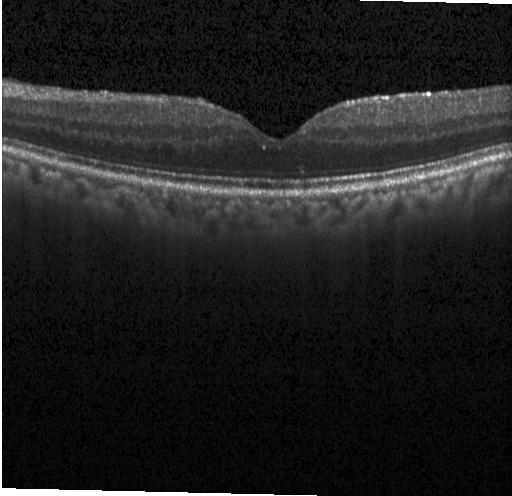

Spectral-domain OCT · retinal OCT cross-section. Impression: no choroidal neovascularization, diabetic macular edema, or drusen.